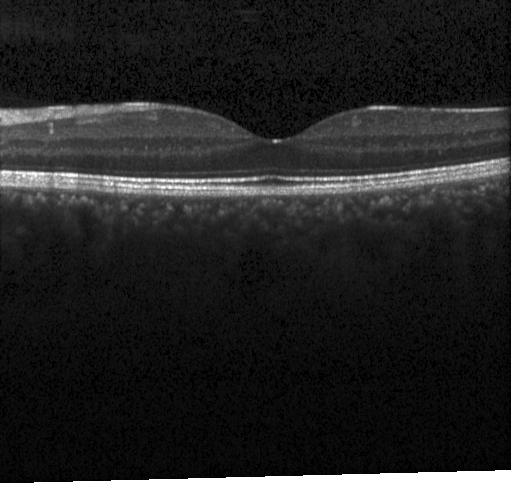 Spectral-domain OCT B-scan: no evidence of CNV, DME, or drusen.